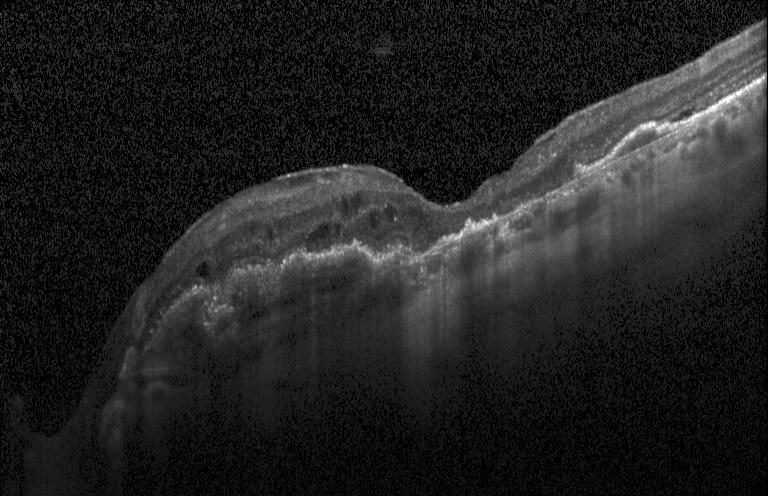 Impression: CNV.